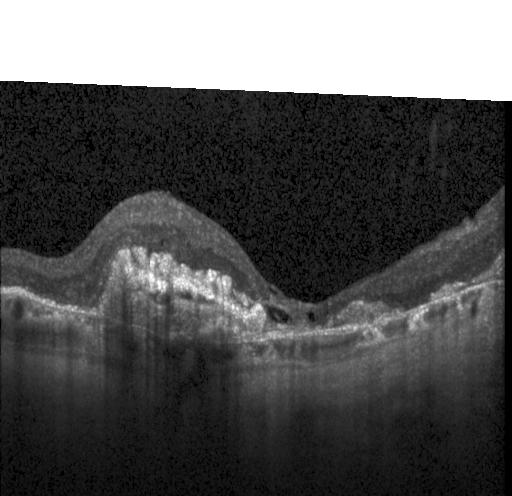 This B-scan demonstrates choroidal neovascularization.